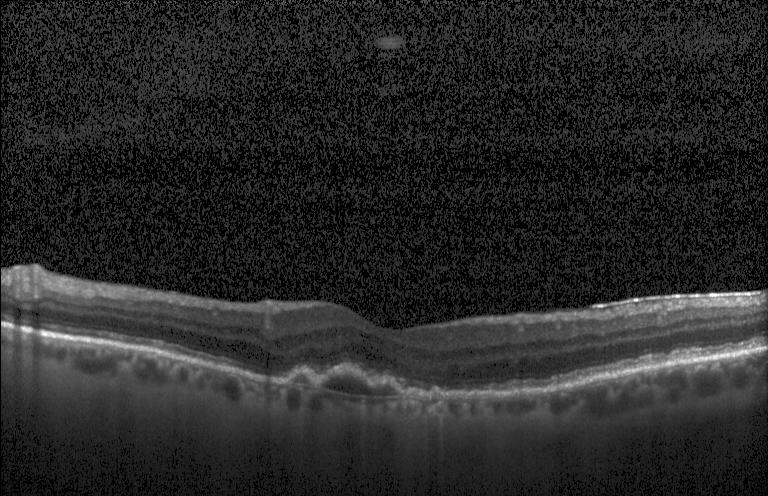 Retinal OCT cross-section showing a choroidal neovascular membrane.